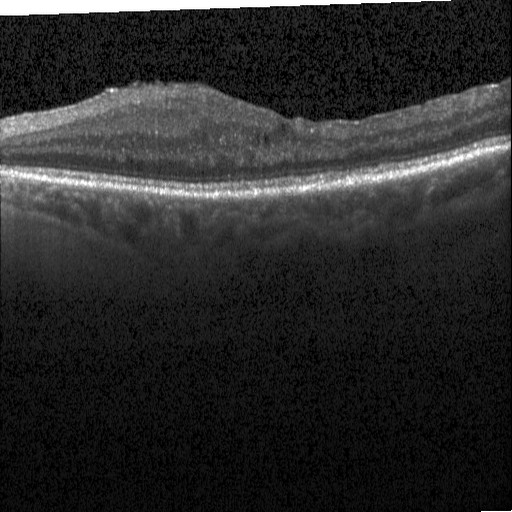
Retinal OCT B-scan. Finding: diabetic macular edema (DME).